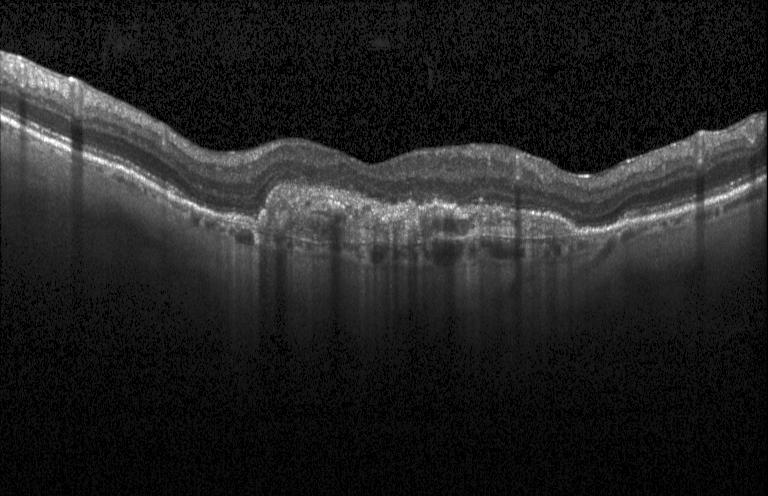

Acquired on a Heidelberg Spectralis. SD-OCT. OCT B-scan. Through the macula — OCT finding: CNV.